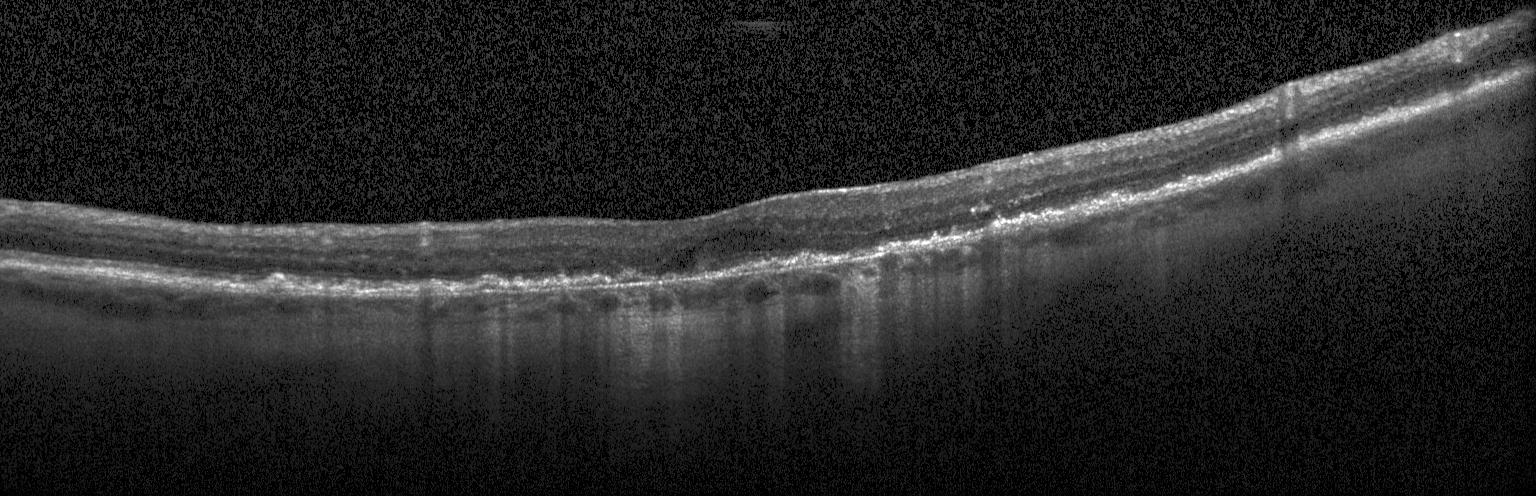

OCT finding: choroidal neovascularization (CNV).